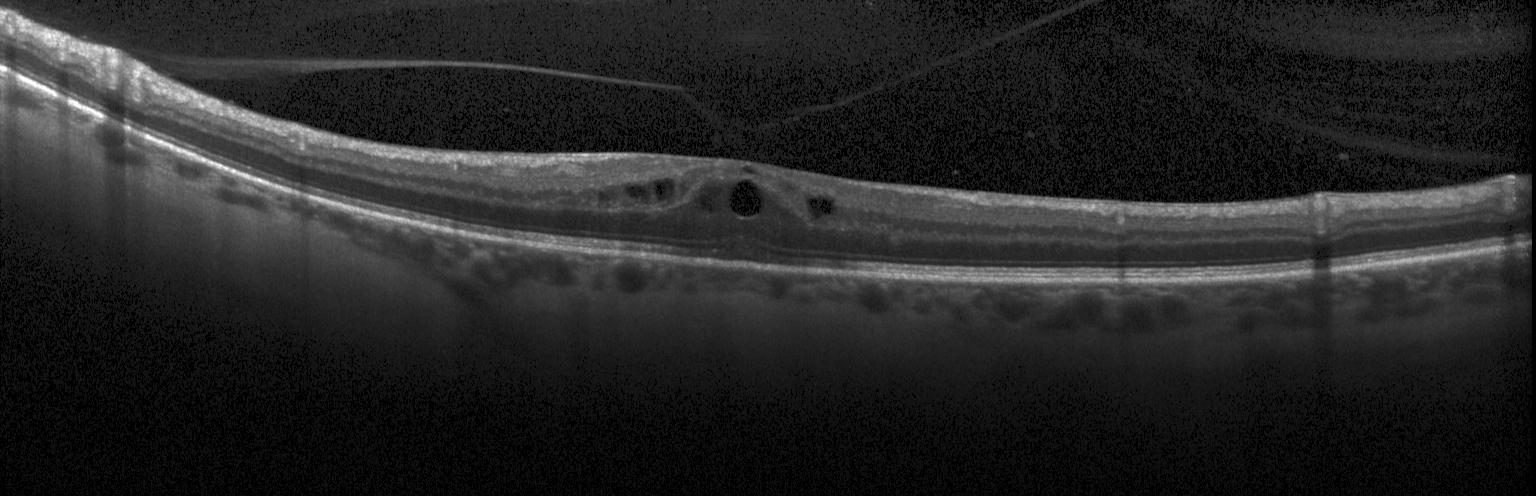 Diabetic macular edema (DME).